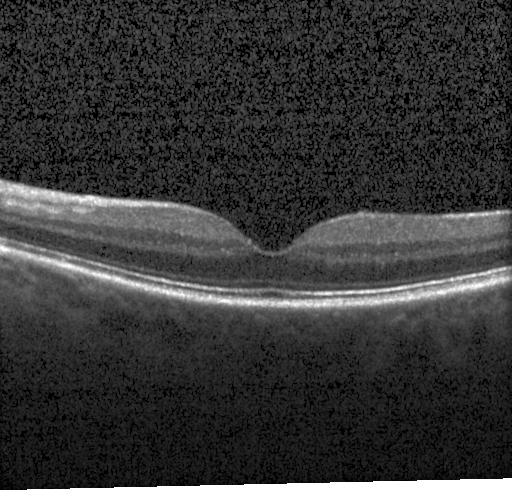
Finding: no choroidal neovascularization, no diabetic macular edema, and no drusen.